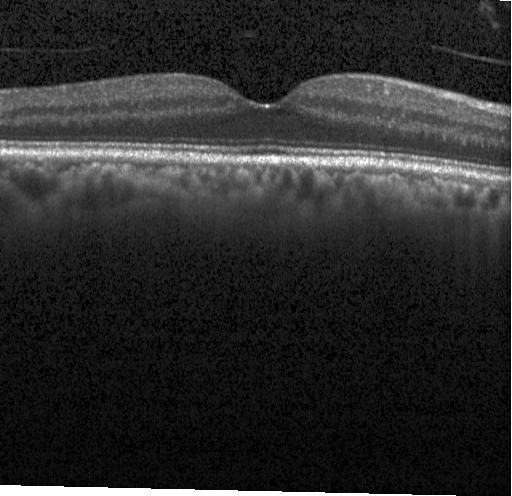

OCT scan showing no choroidal neovascularization, no diabetic macular edema, and no drusen.